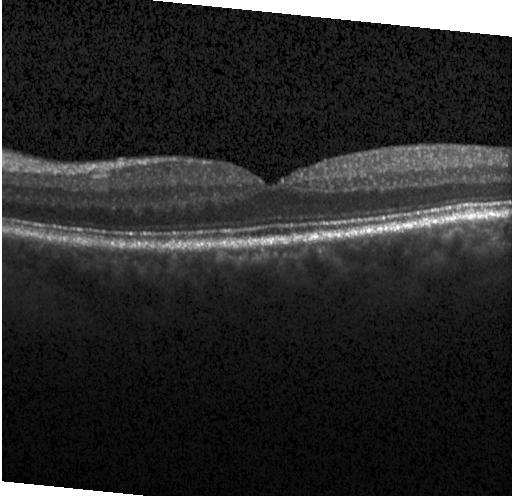
Heidelberg Spectralis OCT system. Optical coherence tomography scan. Centered on the fovea
Finding: no CNV, DME, or drusen.